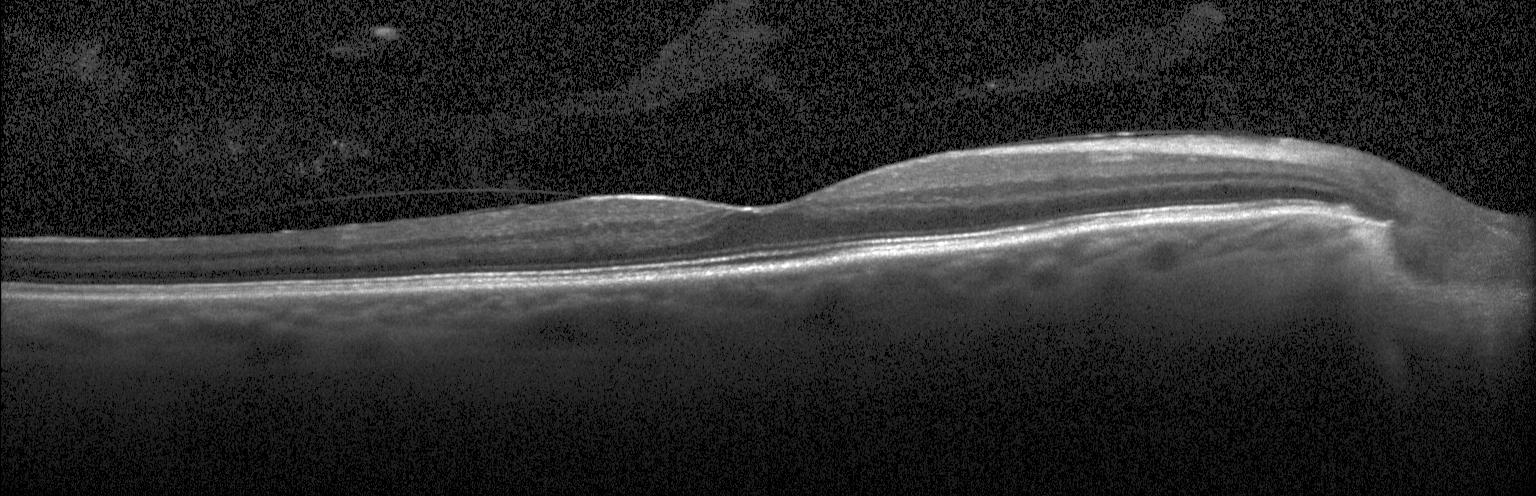
Horizontal scan through the fovea · retinal OCT cross-section · Heidelberg Spectralis
No choroidal neovascularization, diabetic macular edema, or drusen.